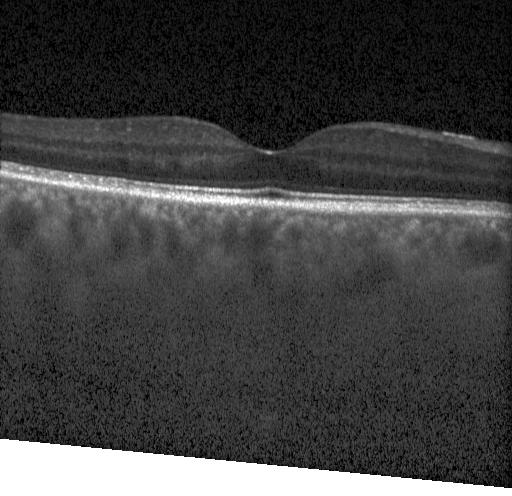
The scan shows no evidence of choroidal neovascularization, diabetic macular edema, or drusen.